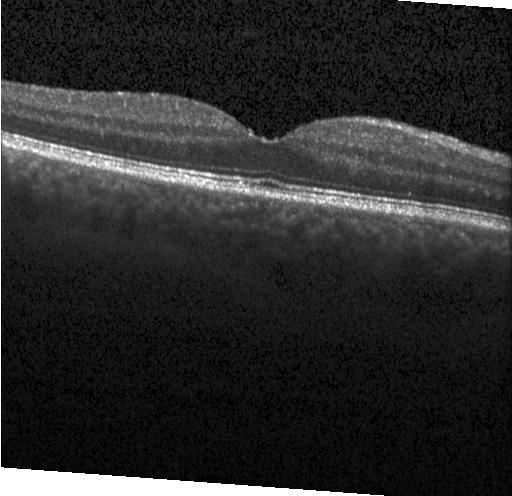

Macular OCT: no evidence of choroidal neovascularization, diabetic macular edema, or drusen.